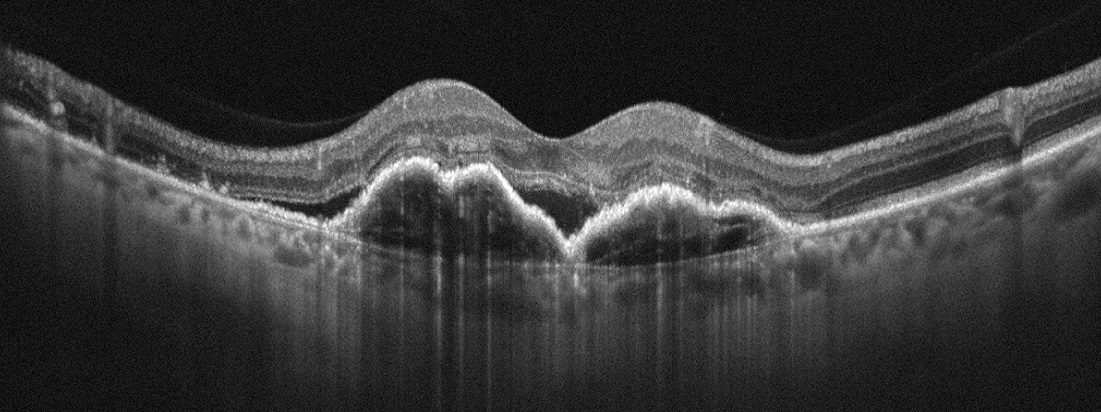

Optical coherence tomography scan — This B-scan demonstrates AMD.